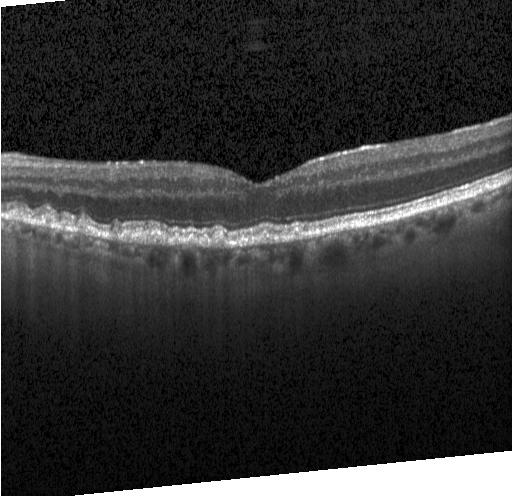

Optical coherence tomography B-scan. Heidelberg Spectralis OCT system — The scan shows drusen.